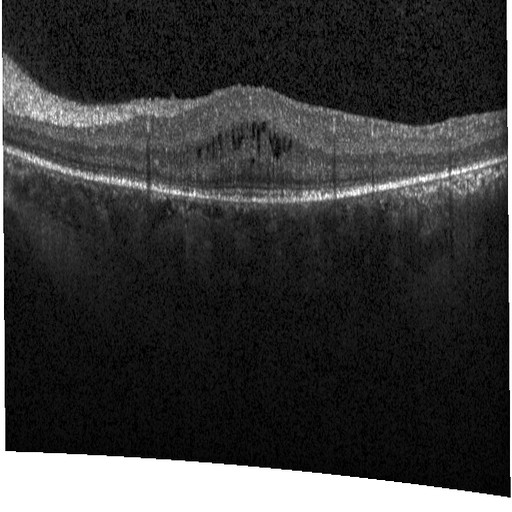

SD-OCT, retinal OCT B-scan. Assessment: diabetic macular edema (DME).